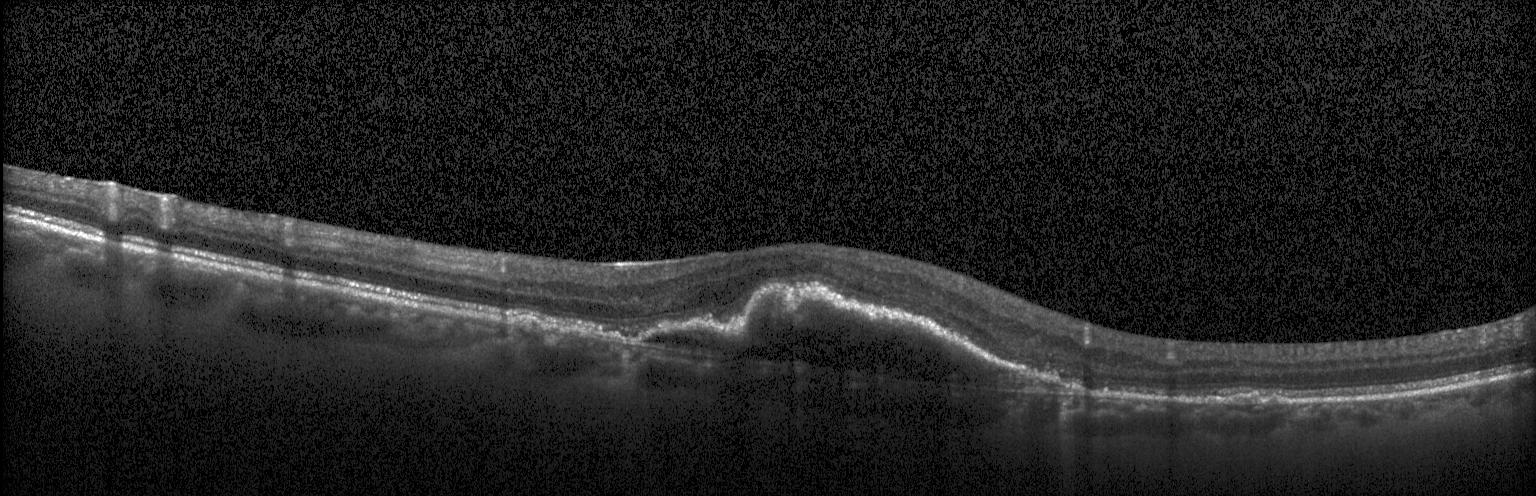

Optical coherence tomography B-scan. Diagnosis: choroidal neovascularization.